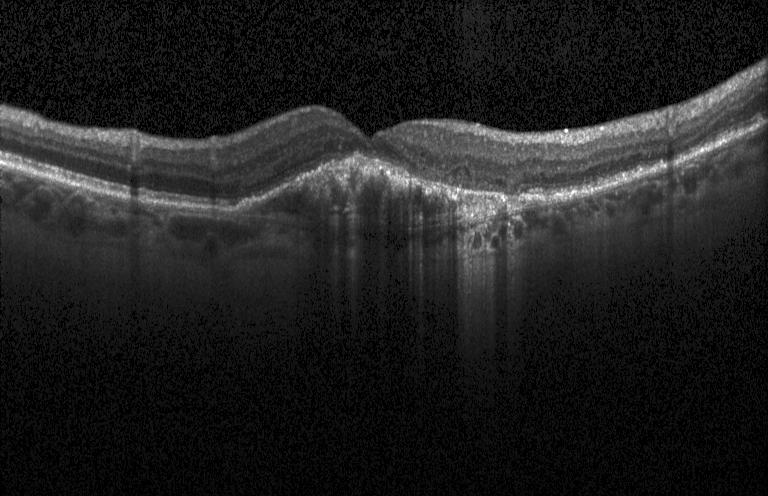 Fovea-centered, Heidelberg Spectralis, retinal OCT B-scan. A choroidal neovascular membrane.